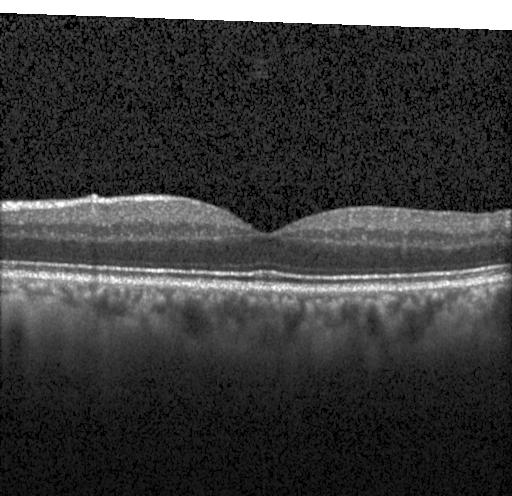
Optical coherence tomography B-scan. Fovea-centered. Heidelberg Spectralis. OCT finding: no CNV, no DME, and no drusen.